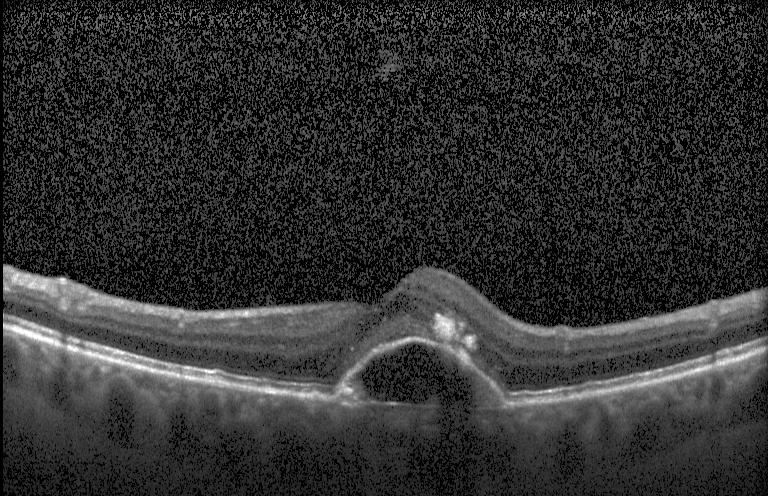 Impression: choroidal neovascularization (CNV).